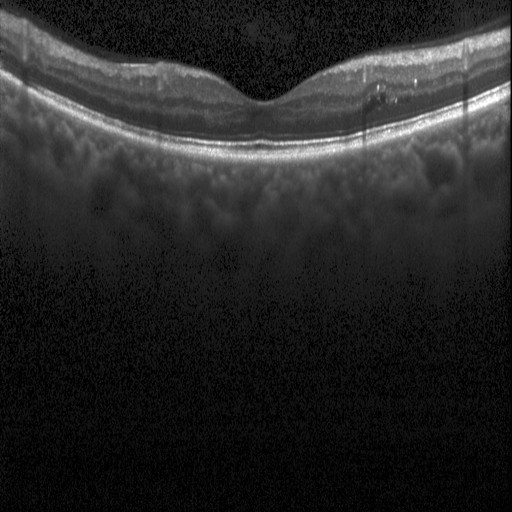

Spectral-domain optical coherence tomography; fovea-centered; OCT line scan; acquired on a Heidelberg Spectralis
Finding: diabetic macular edema.